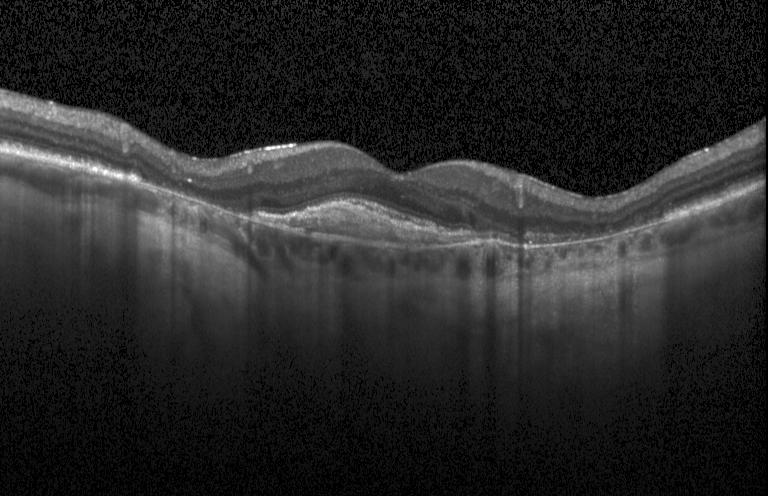 SD-OCT · OCT B-scan — OCT finding: a choroidal neovascular membrane.